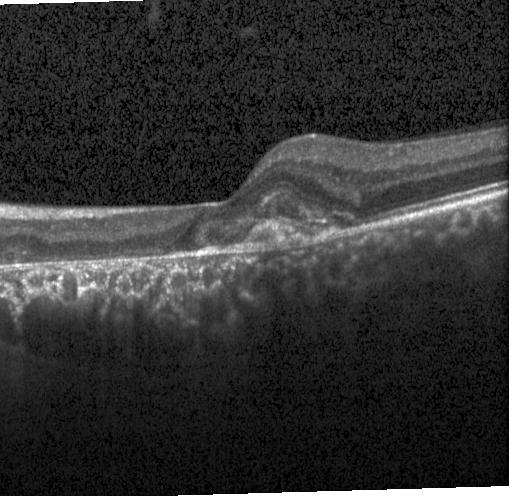 Retinal OCT cross-section. Diagnosis: a choroidal neovascular membrane.